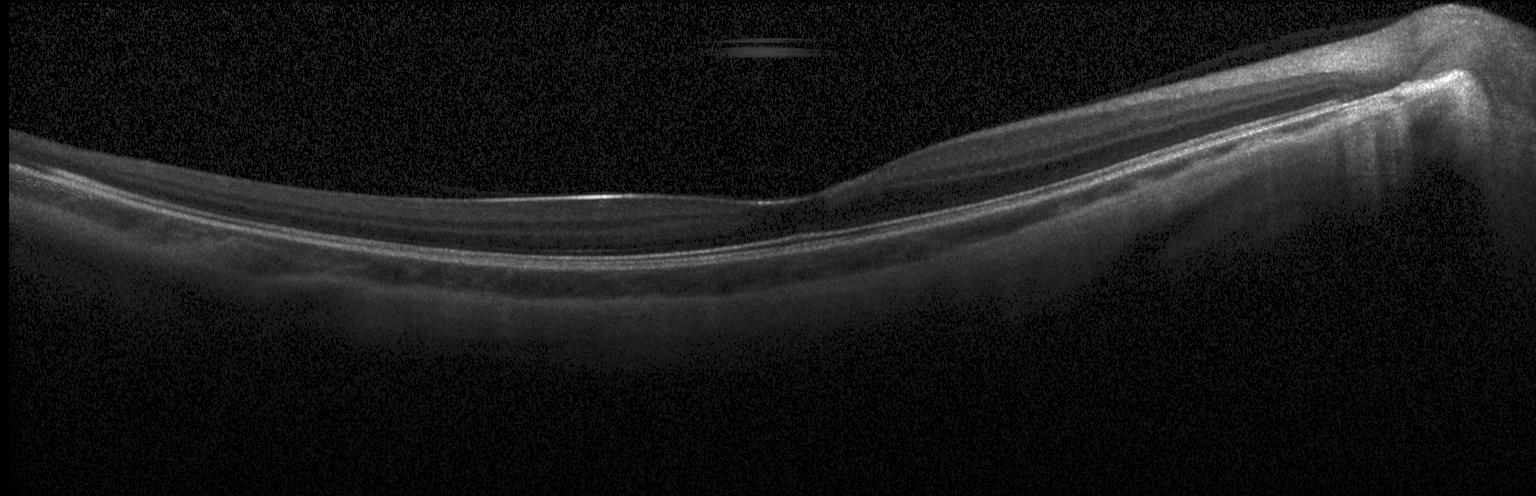

SD-OCT · centered on the fovea · optical coherence tomography scan.
Impression: no evidence of choroidal neovascularization, diabetic macular edema, or drusen.